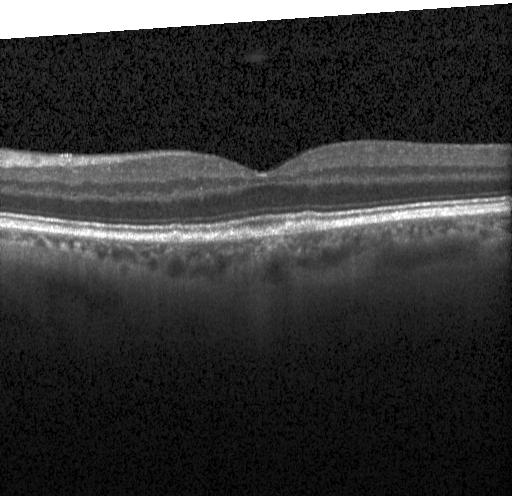
Impression: multiple drusen.